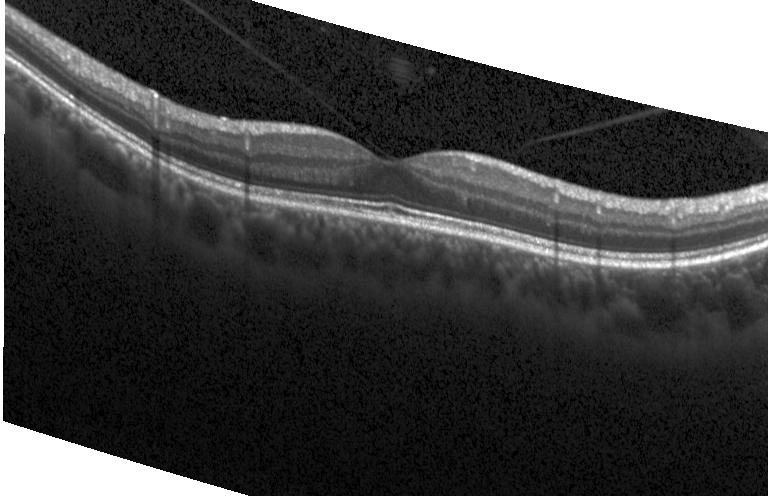 Instrument: Heidelberg Spectralis. Retinal OCT B-scan. Assessment: no evidence of CNV, DME, or drusen.